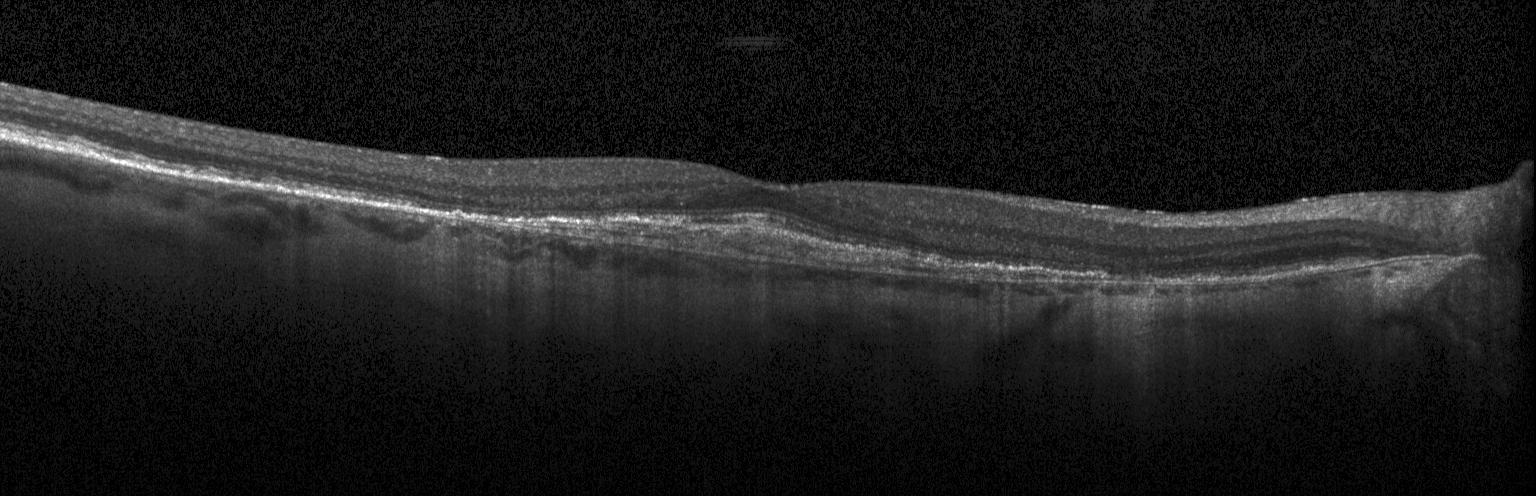

Spectral-domain OCT; optical coherence tomography B-scan; centered on the fovea; Heidelberg Spectralis OCT system
This B-scan demonstrates choroidal neovascularization (CNV).